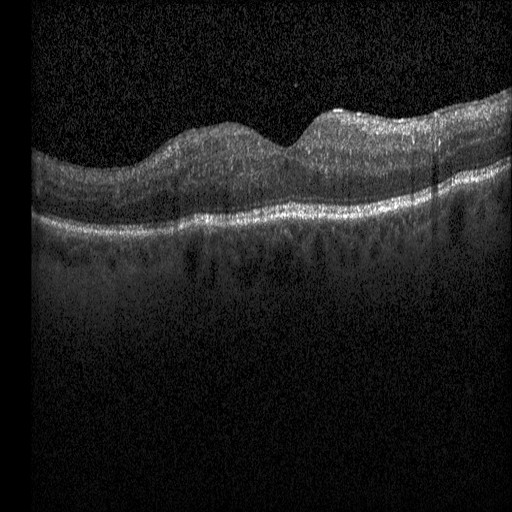

Dx: DME.